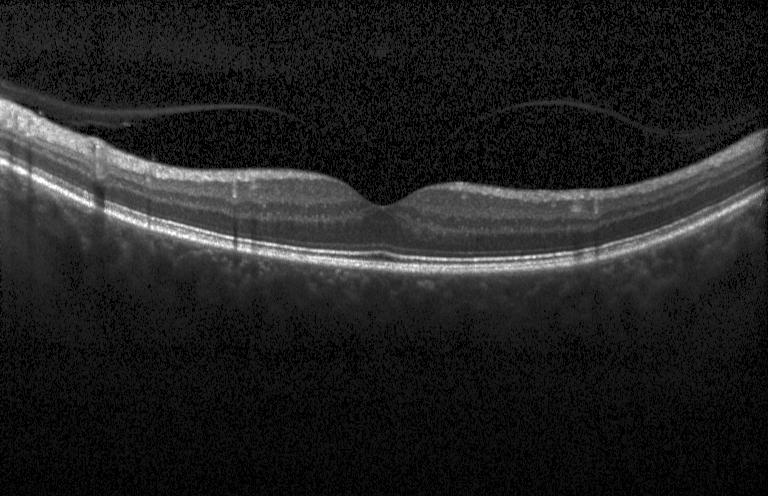
OCT finding: no CNV, DME, or drusen.